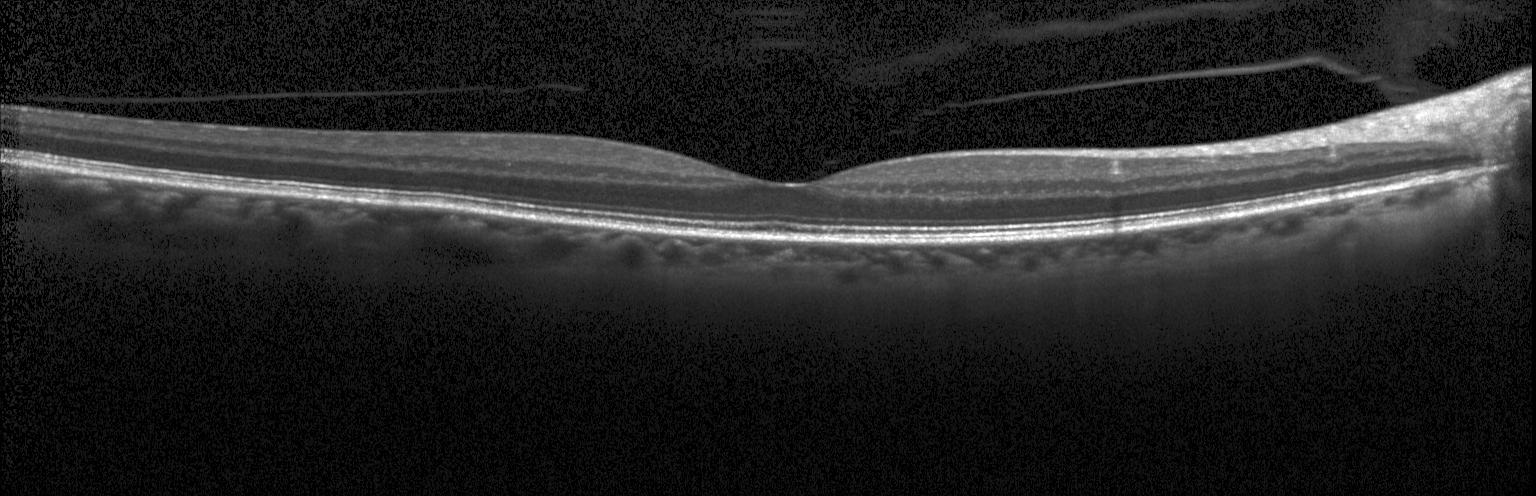

OCT line scan — Macular OCT: neither choroidal neovascularization, diabetic macular edema, nor drusen.